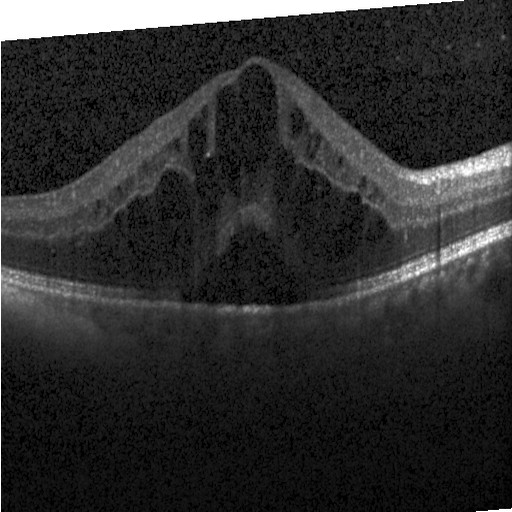
The scan shows DME.